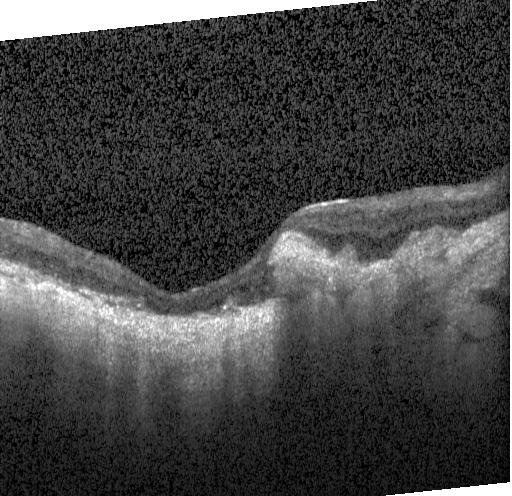
OCT B-scan; Heidelberg Spectralis OCT system; SD-OCT; horizontal scan through the fovea — Finding: choroidal neovascularization.